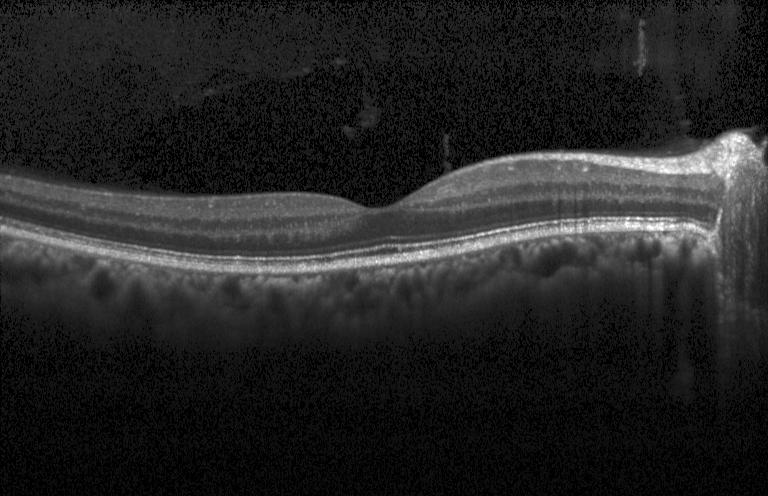 Assessment: no choroidal neovascularization, no diabetic macular edema, and no drusen.